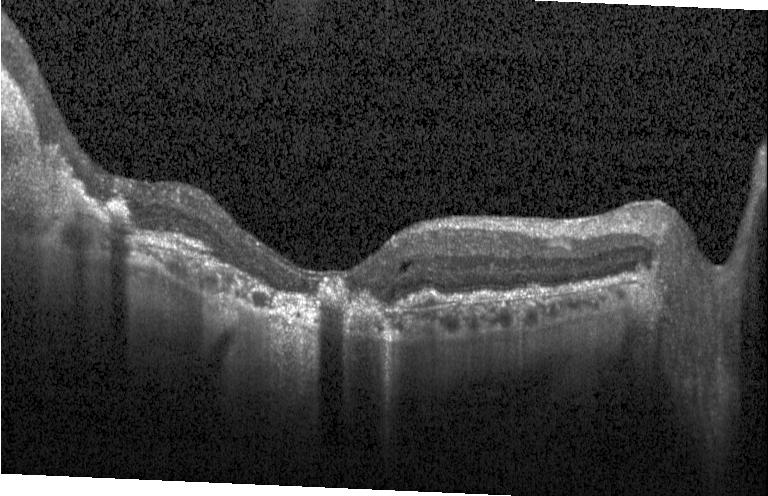

Finding: a choroidal neovascular membrane.